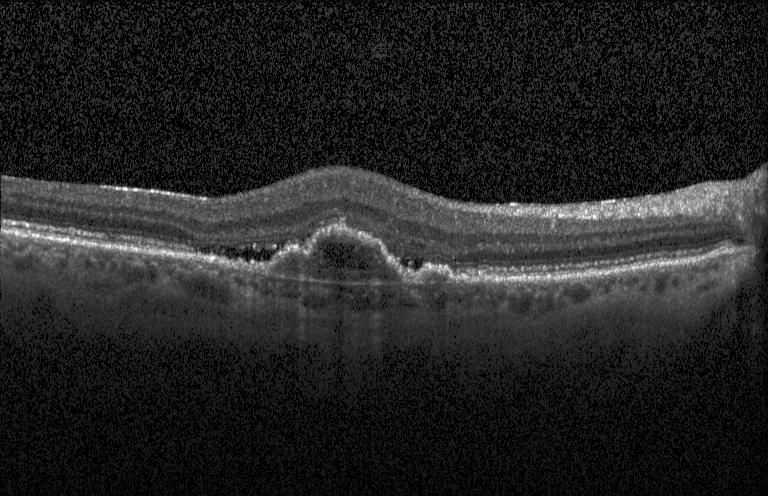 Retinal OCT B-scan; acquired on a Heidelberg Spectralis; spectral-domain OCT
Finding: a choroidal neovascular membrane.